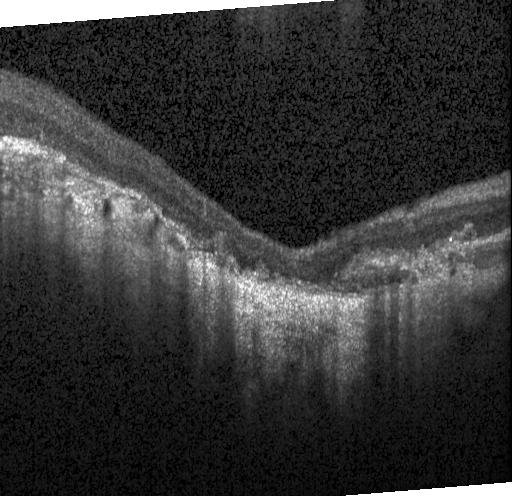

OCT B-scan showing CNV.